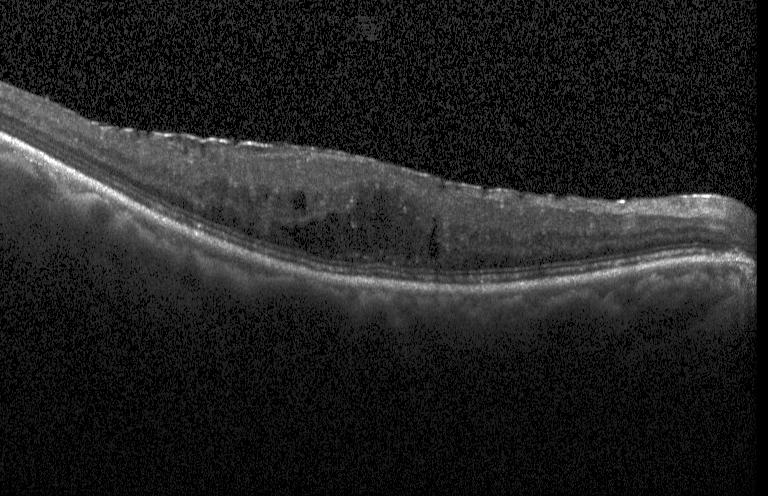 Optical coherence tomography scan, spectral-domain optical coherence tomography, through the macula, Heidelberg Spectralis OCT system — Macular OCT: diabetic macular edema.